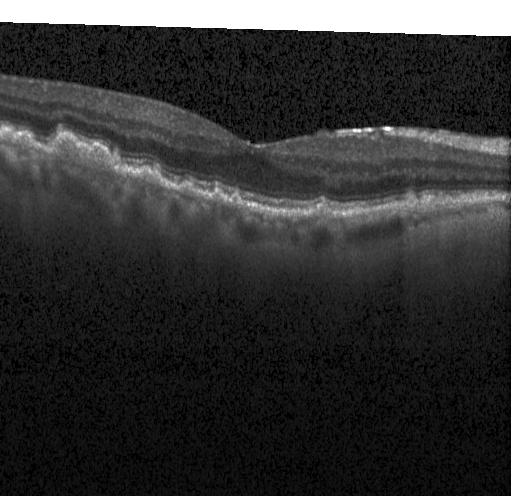

Retinal OCT cross-section, Heidelberg Spectralis OCT system
Assessment: sub-RPE drusenoid deposits.